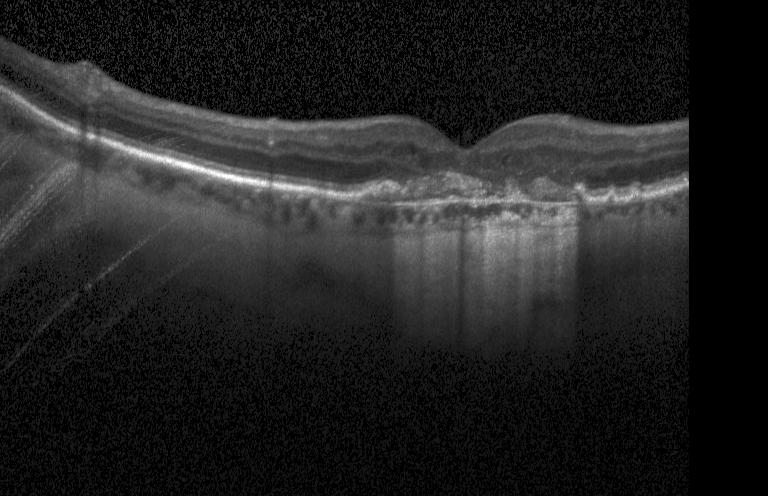

Spectral-domain OCT B-scan: choroidal neovascularization.